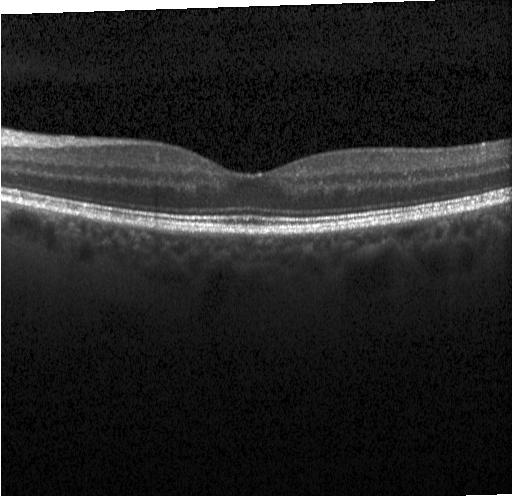

OCT line scan
Finding: neither CNV, DME, nor drusen.